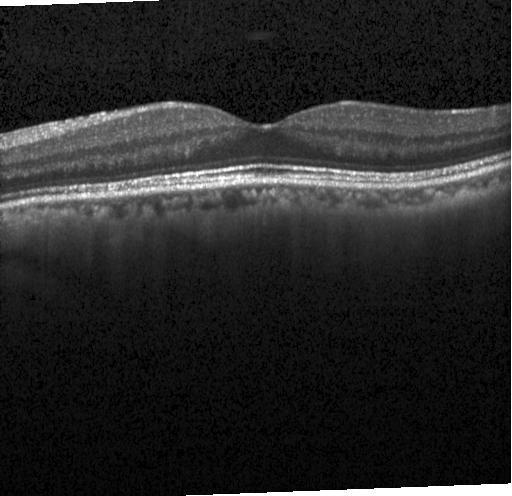
Finding: neither CNV, DME, nor drusen.